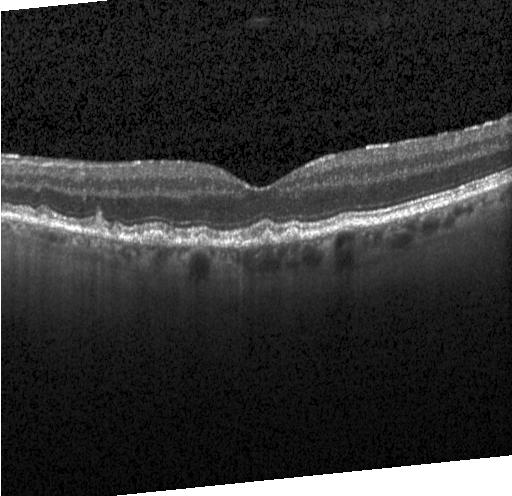
Optical coherence tomography B-scan — Finding: multiple drusen.